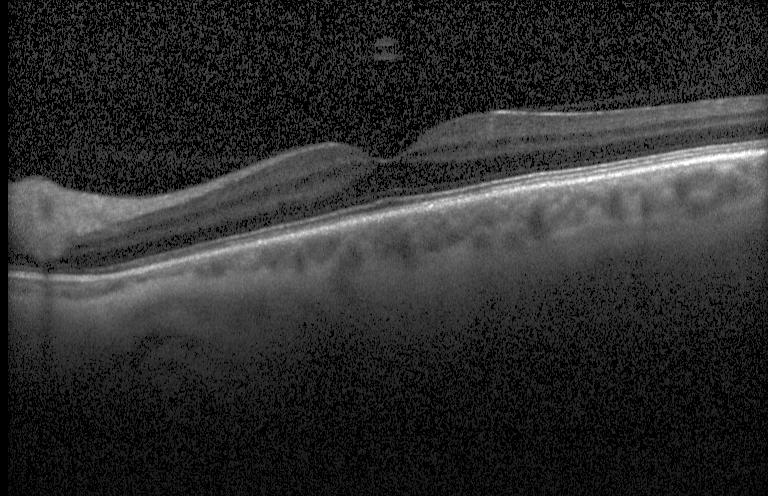

OCT scan showing neither choroidal neovascularization, diabetic macular edema, nor drusen.